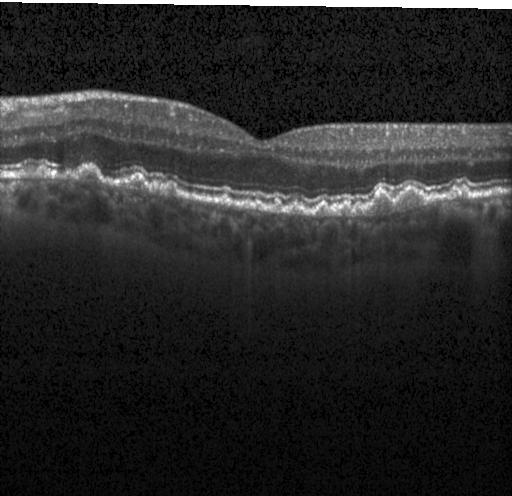
Acquired on a Heidelberg Spectralis. Spectral-domain OCT. Optical coherence tomography scan. This B-scan demonstrates sub-RPE drusenoid deposits.